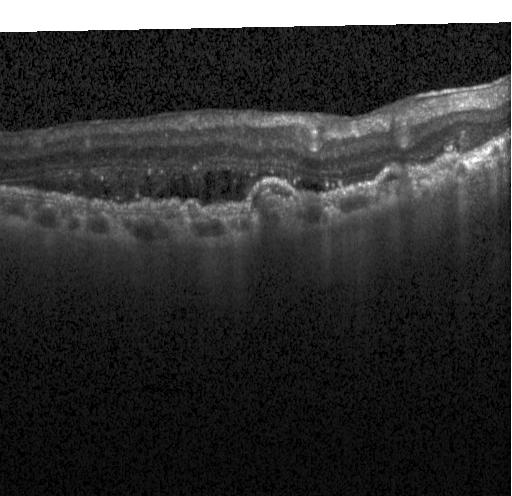

Horizontal scan through the fovea, spectral-domain optical coherence tomography, optical coherence tomography scan. Finding: a choroidal neovascular membrane.